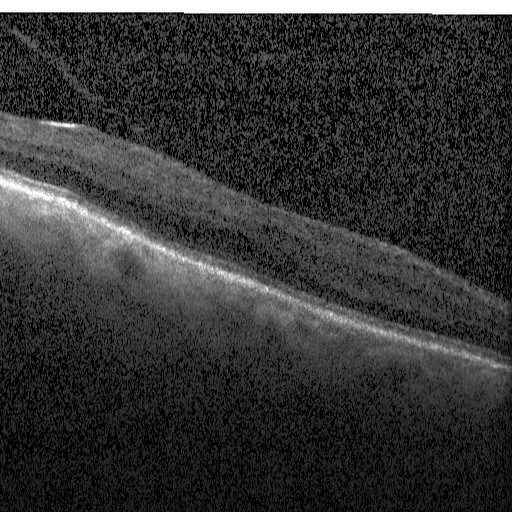 OCT B-scan, Heidelberg Spectralis, horizontal scan through the fovea.
Diagnosis: diabetic macular edema.